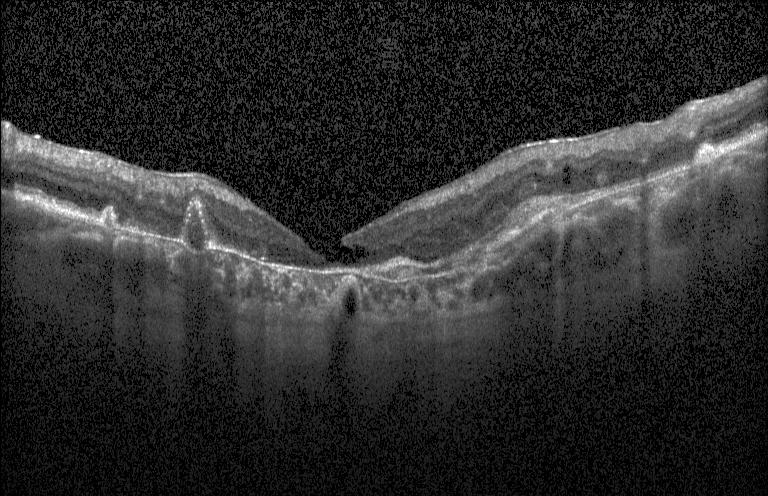
Dx: choroidal neovascularization.